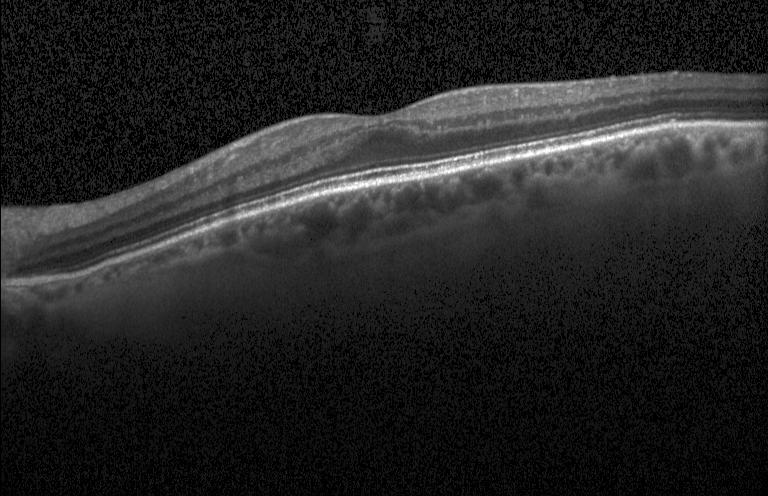

Fovea-centered · optical coherence tomography scan. Impression: neither CNV, DME, nor drusen.